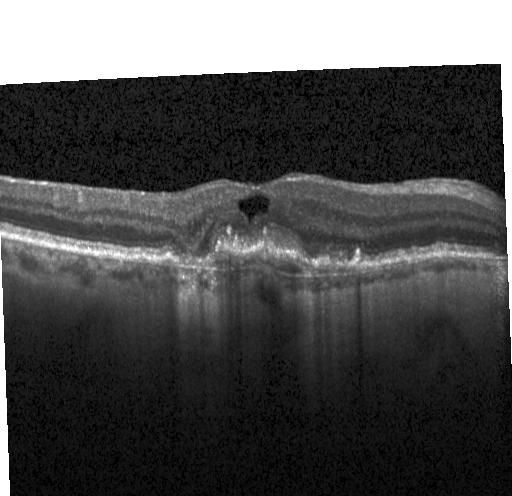

Retinal OCT cross-section; macular scan.
The scan shows a choroidal neovascular membrane.